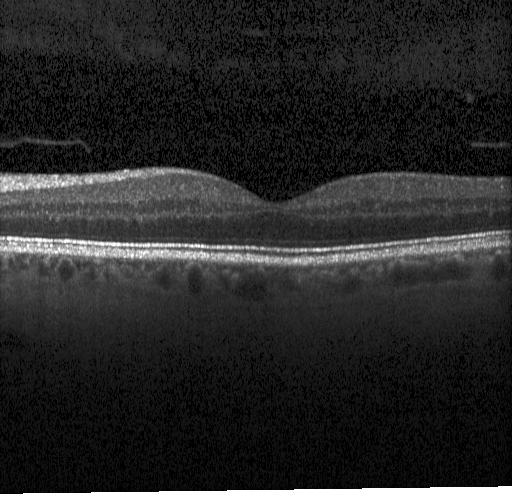 Macular scan. Instrument: Heidelberg Spectralis. OCT line scan.
The scan shows no evidence of CNV, DME, or drusen.